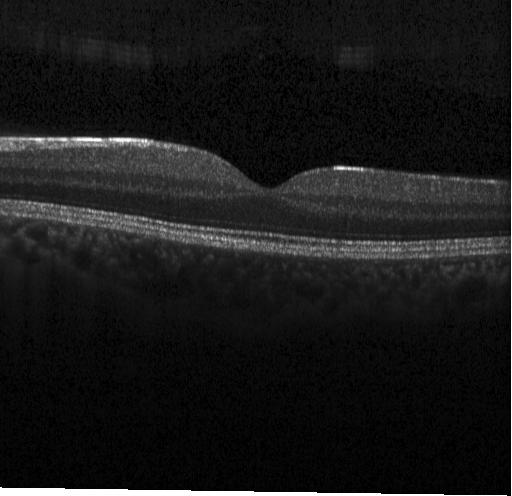
Spectral-domain OCT · acquired on a Heidelberg Spectralis · retinal OCT B-scan — Neither CNV, DME, nor drusen.